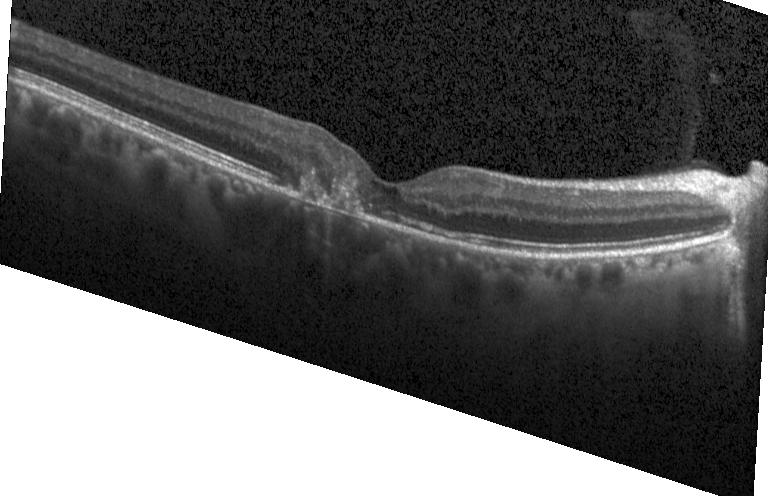 Retinal OCT cross-section — Diagnosis: a choroidal neovascular membrane.